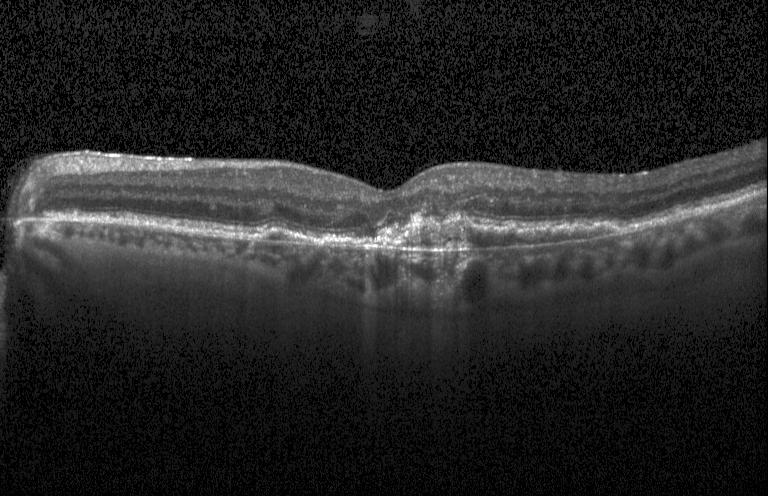
OCT finding: a choroidal neovascular membrane.